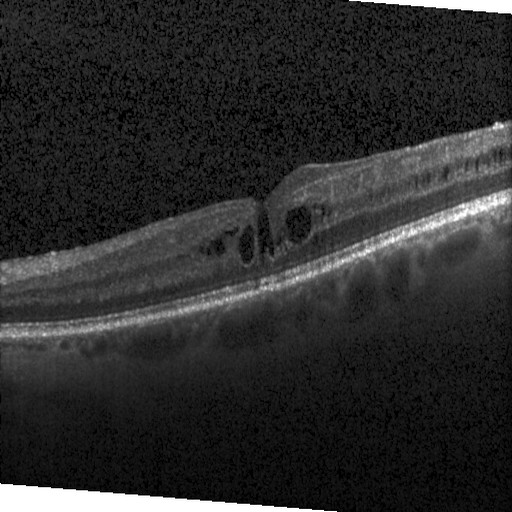
Centered on the fovea · retinal OCT B-scan
The scan shows diabetic macular edema.